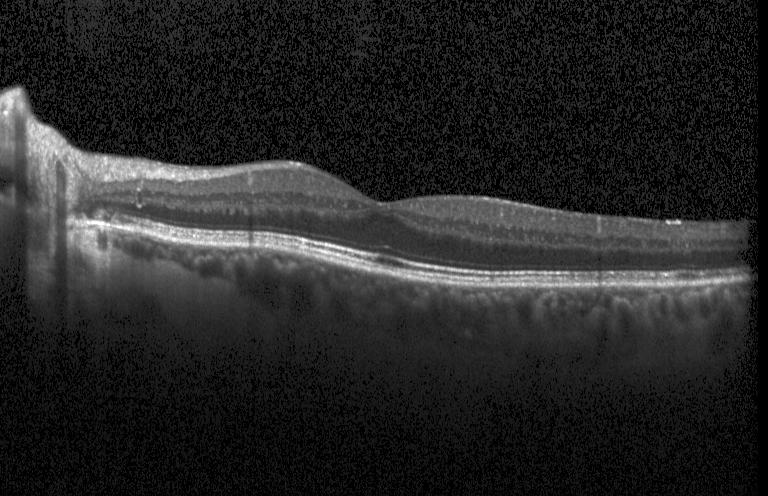

Retinal OCT B-scan, spectral-domain optical coherence tomography, Heidelberg Spectralis. Dx: no CNV, DME, or drusen.